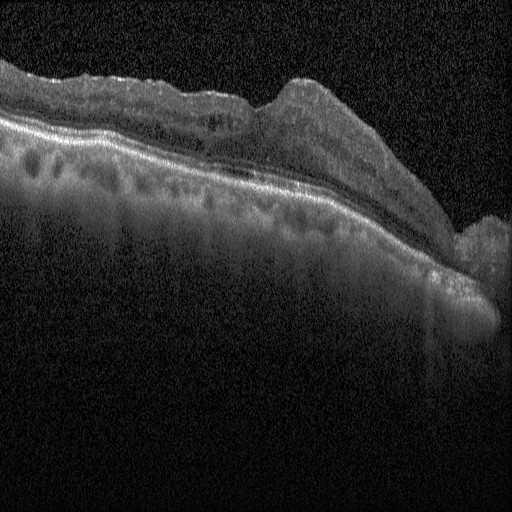 Heidelberg Spectralis, fovea-centered, OCT B-scan, SD-OCT. Macular OCT: diabetic macular edema (DME).